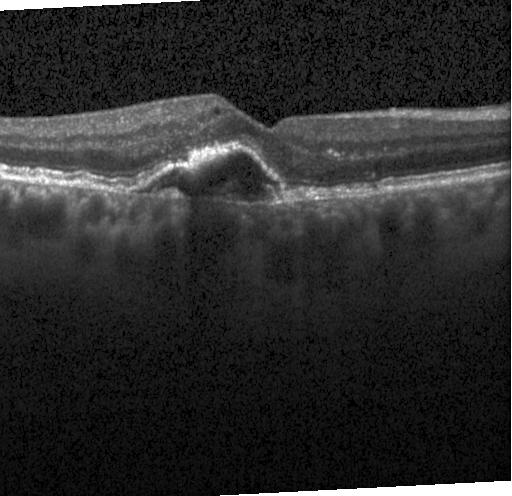
SD-OCT, optical coherence tomography B-scan, acquired on a Heidelberg Spectralis, through the macula. Macular OCT: a choroidal neovascular membrane.